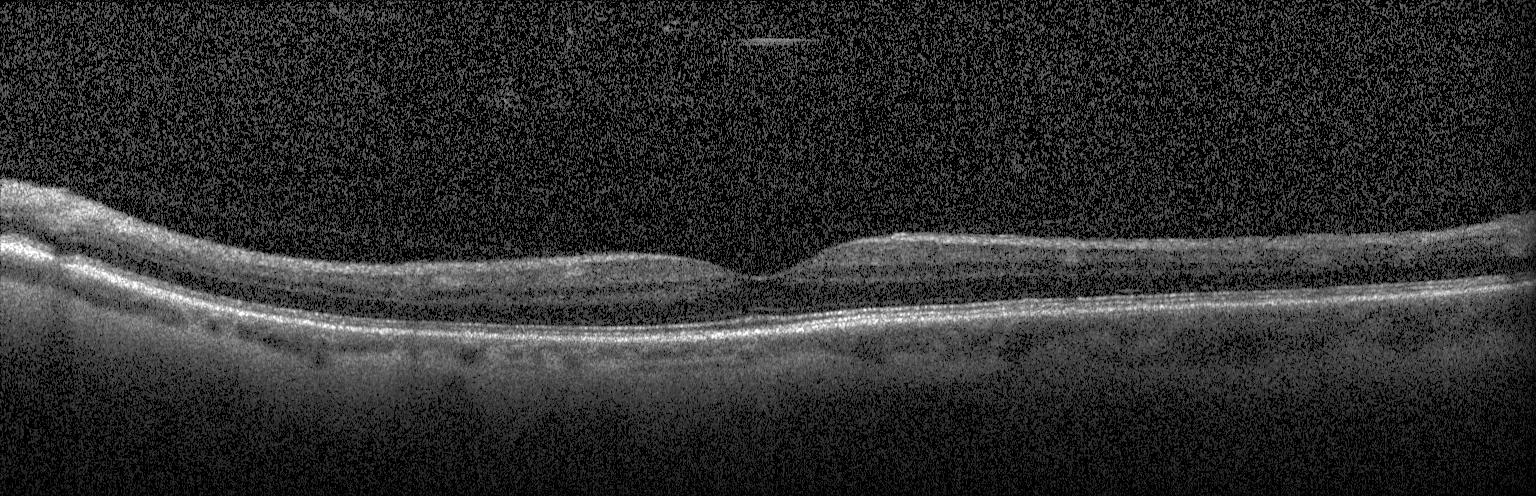 Diagnosis: neither CNV, DME, nor drusen.